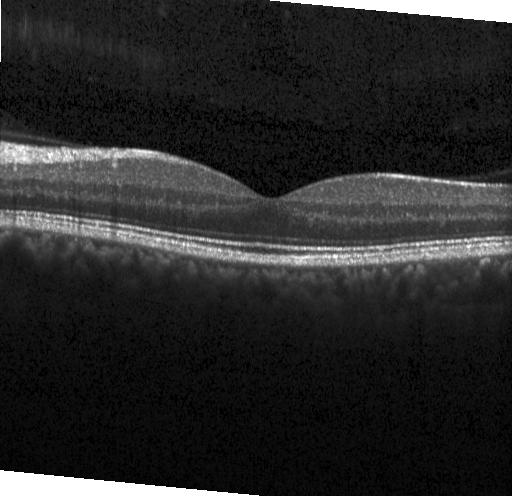 Heidelberg Spectralis OCT system; optical coherence tomography scan.
Impression: no choroidal neovascularization, no diabetic macular edema, and no drusen.